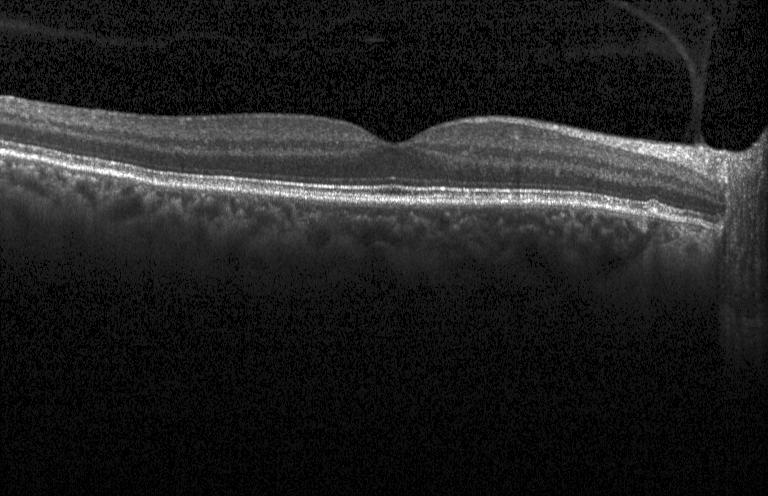
Fovea-centered; SD-OCT; instrument: Heidelberg Spectralis; optical coherence tomography scan — The scan shows multiple drusen.